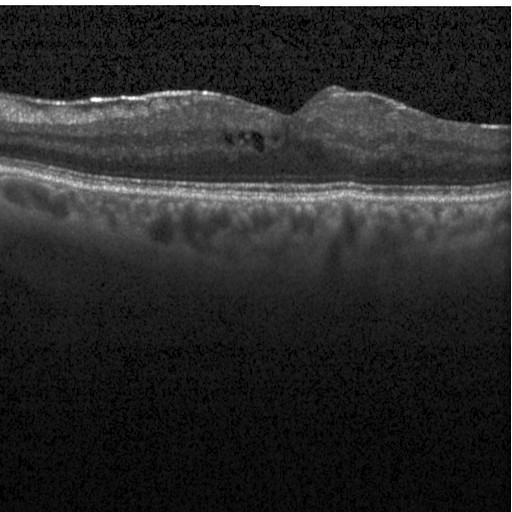

Spectral-domain optical coherence tomography · horizontal scan through the fovea · acquired on a Heidelberg Spectralis · optical coherence tomography B-scan.
DME.